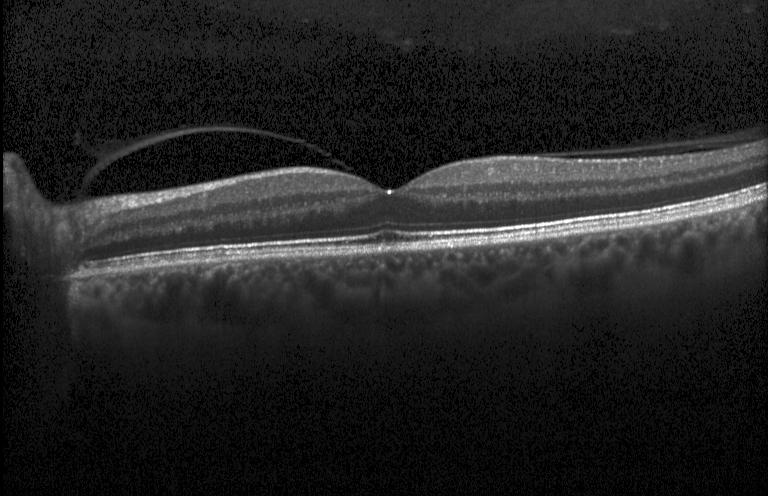

The scan shows no CNV, no DME, and no drusen.